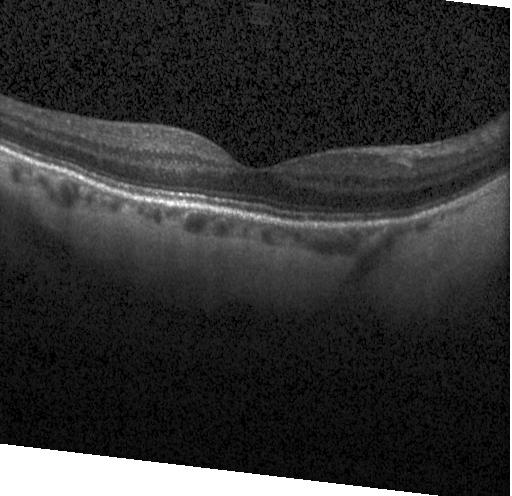
Acquired on a Heidelberg Spectralis, OCT line scan.
Finding: no choroidal neovascularization, no diabetic macular edema, and no drusen.